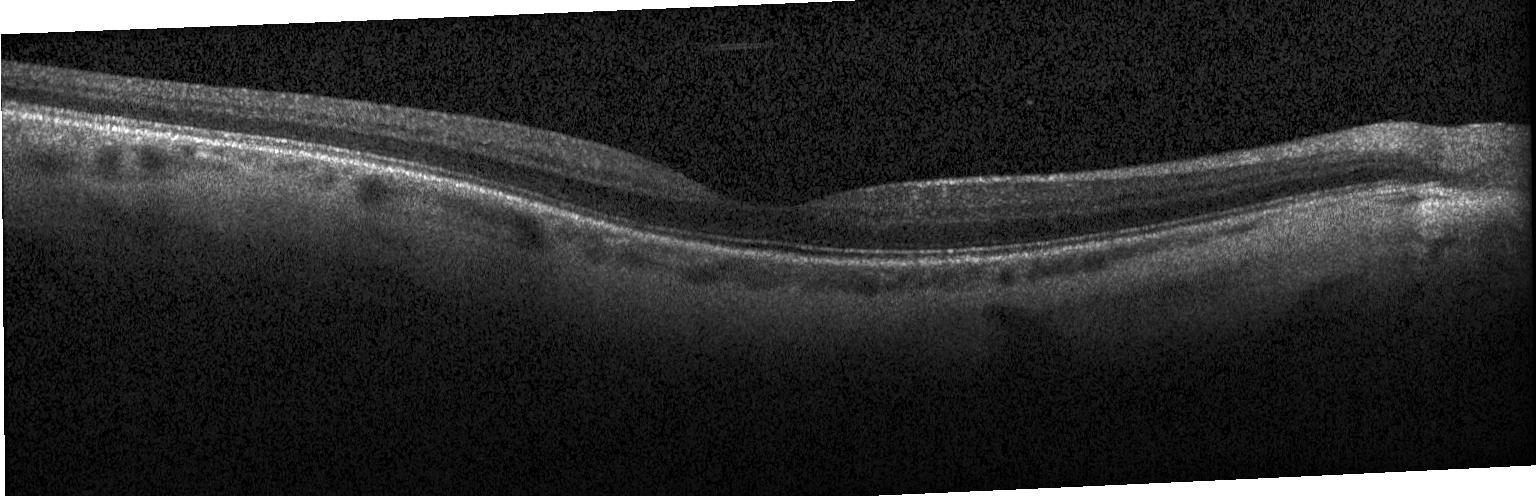

Fovea-centered · spectral-domain OCT · retinal OCT cross-section
Macular OCT: neither CNV, DME, nor drusen.